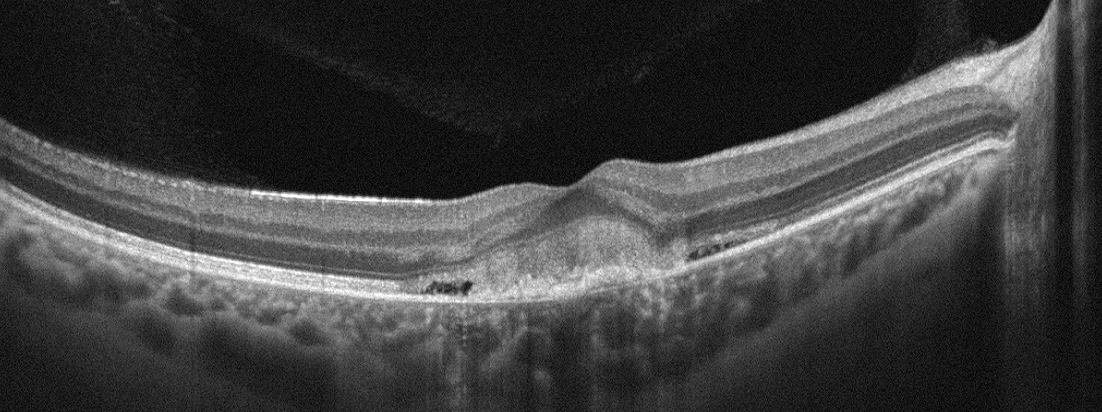
OCT B-scan — Impression: AMD.